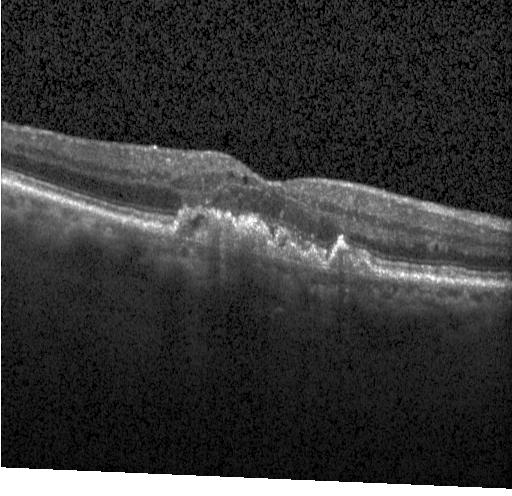 Macular OCT demonstrating choroidal neovascularization.